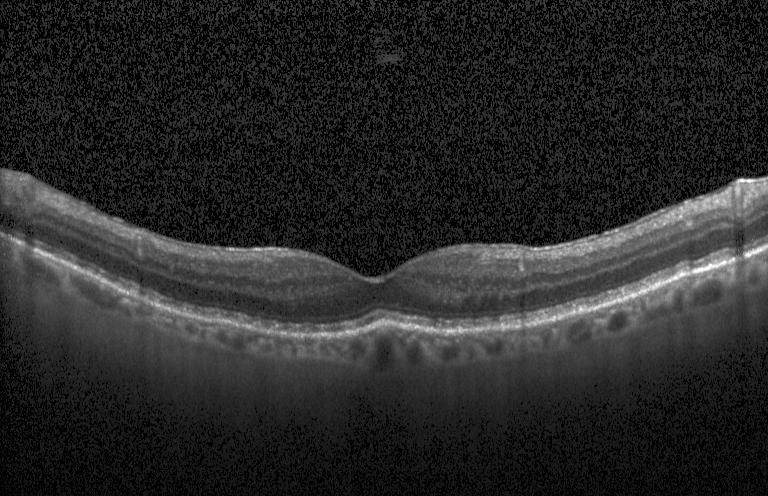 Retinal OCT B-scan. Finding: no evidence of CNV, DME, or drusen.